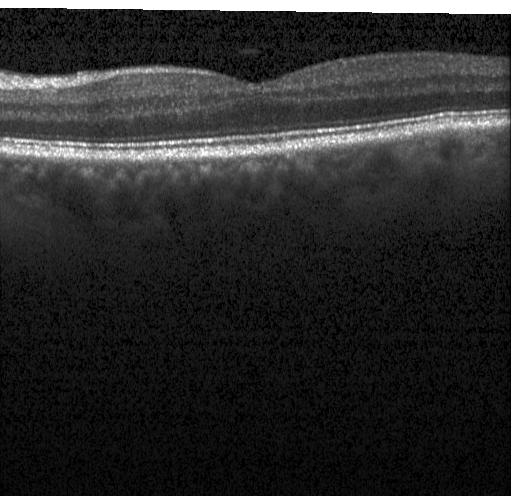
OCT finding: no evidence of choroidal neovascularization, diabetic macular edema, or drusen.